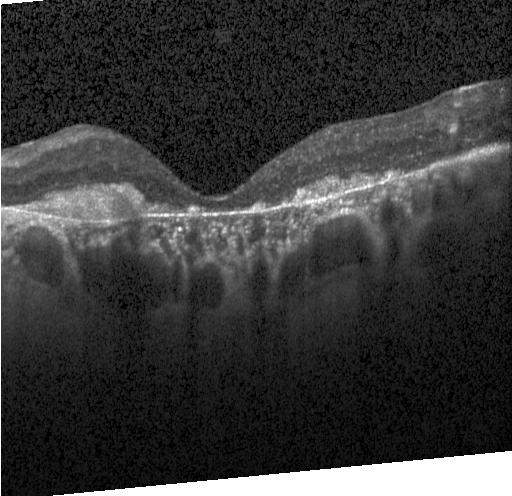
OCT line scan · instrument: Heidelberg Spectralis · SD-OCT · fovea-centered
Impression: choroidal neovascularization (CNV).